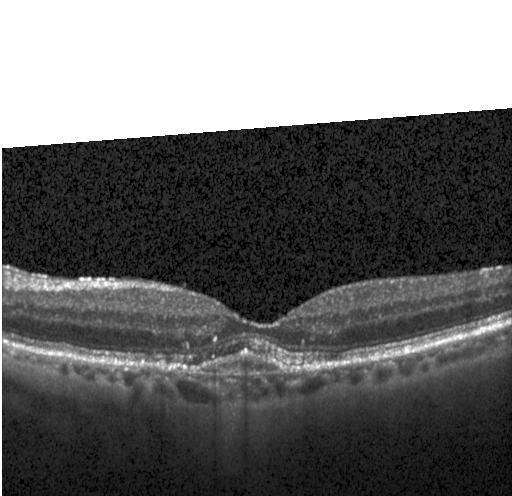
OCT line scan — OCT finding: CNV.